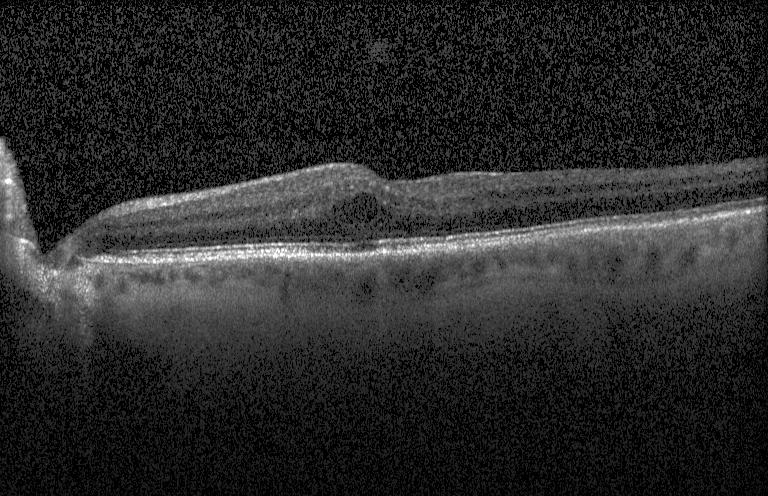 OCT scan showing diabetic macular edema.